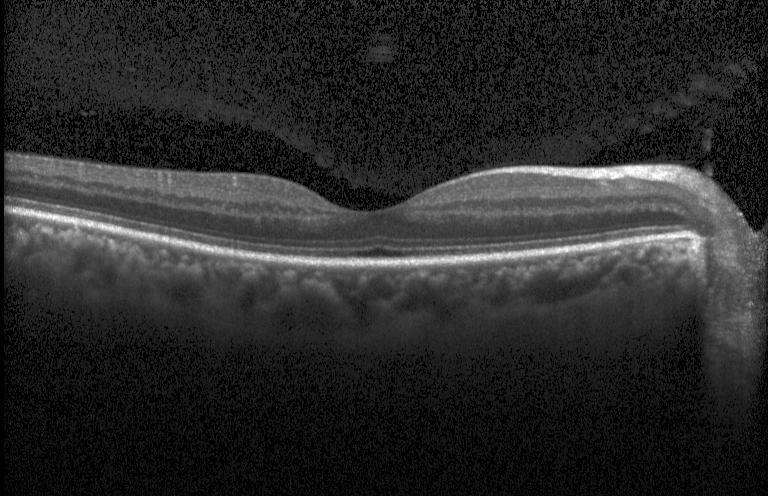

Retinal OCT cross-section, SD-OCT.
Diagnosis: no choroidal neovascularization, no diabetic macular edema, and no drusen.